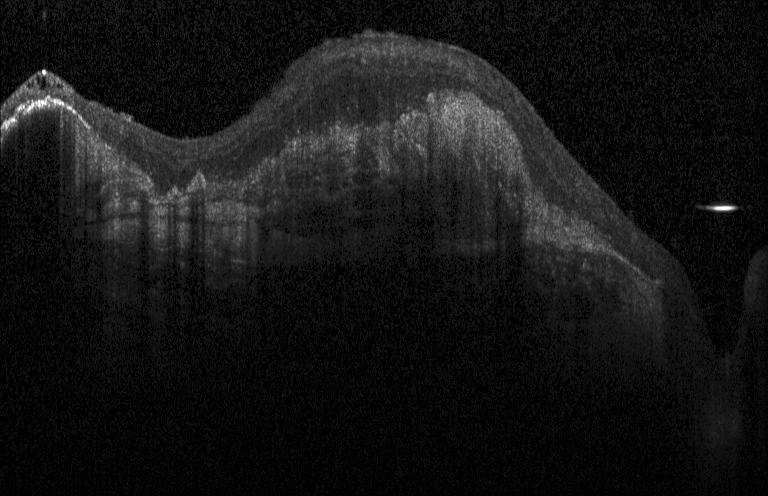
Spectral-domain OCT B-scan: a choroidal neovascular membrane.